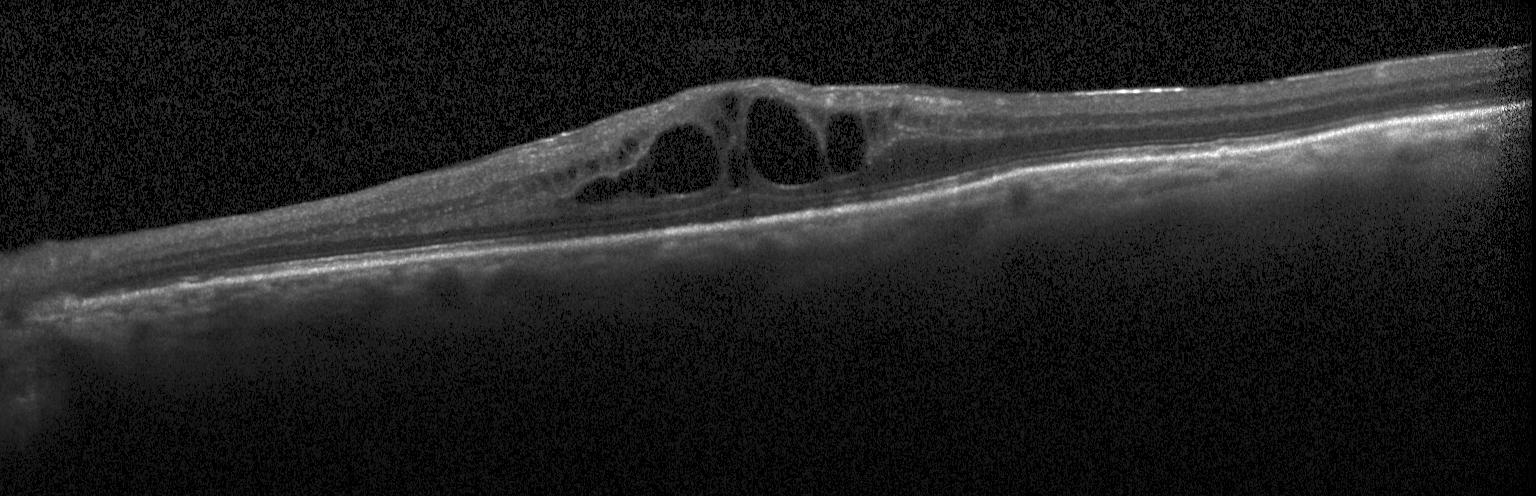 Through the macula; OCT B-scan; spectral-domain optical coherence tomography. Impression: diabetic macular edema (DME).